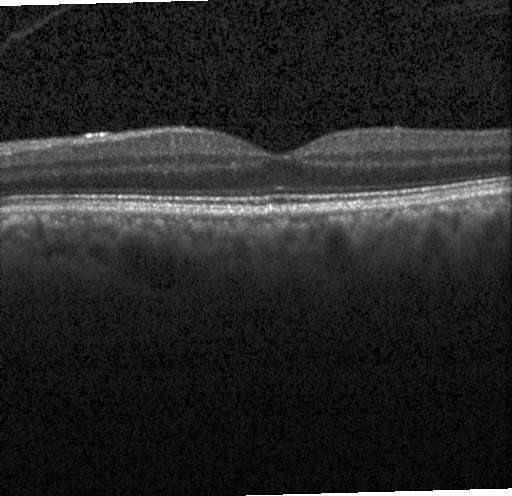
Spectral-domain optical coherence tomography; macular scan; acquired on a Heidelberg Spectralis; retinal OCT cross-section.
Impression: no evidence of CNV, DME, or drusen.